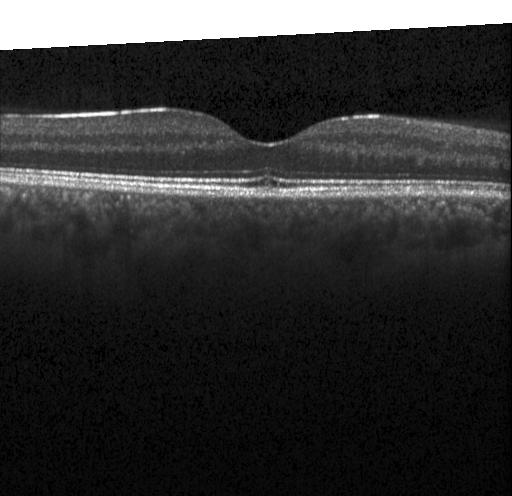

OCT B-scan showing no evidence of choroidal neovascularization, diabetic macular edema, or drusen.